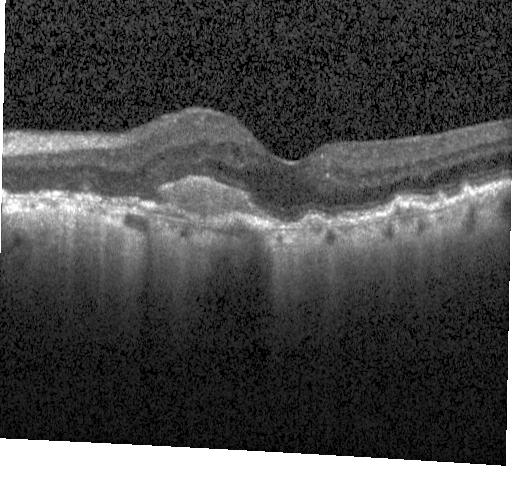
The scan shows CNV.